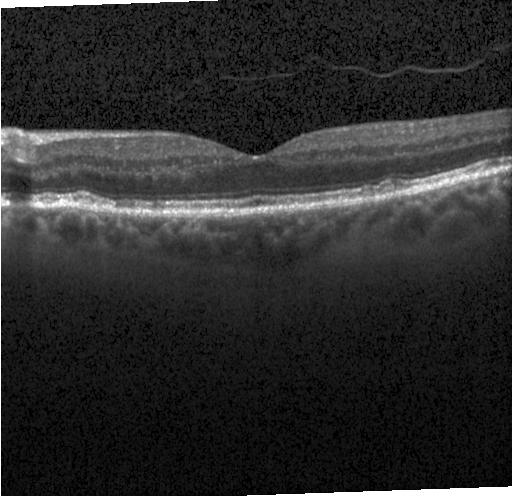

Optical coherence tomography B-scan
Impression: drusen.